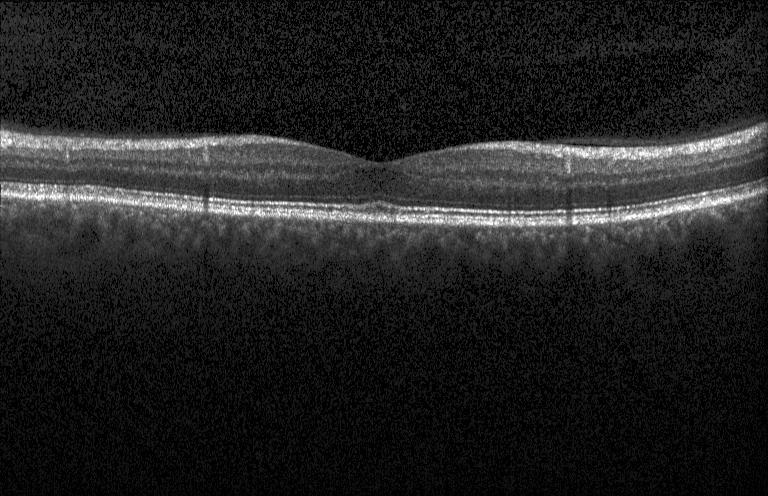
Optical coherence tomography scan, SD-OCT, instrument: Heidelberg Spectralis, macular scan — OCT finding: no CNV, DME, or drusen.